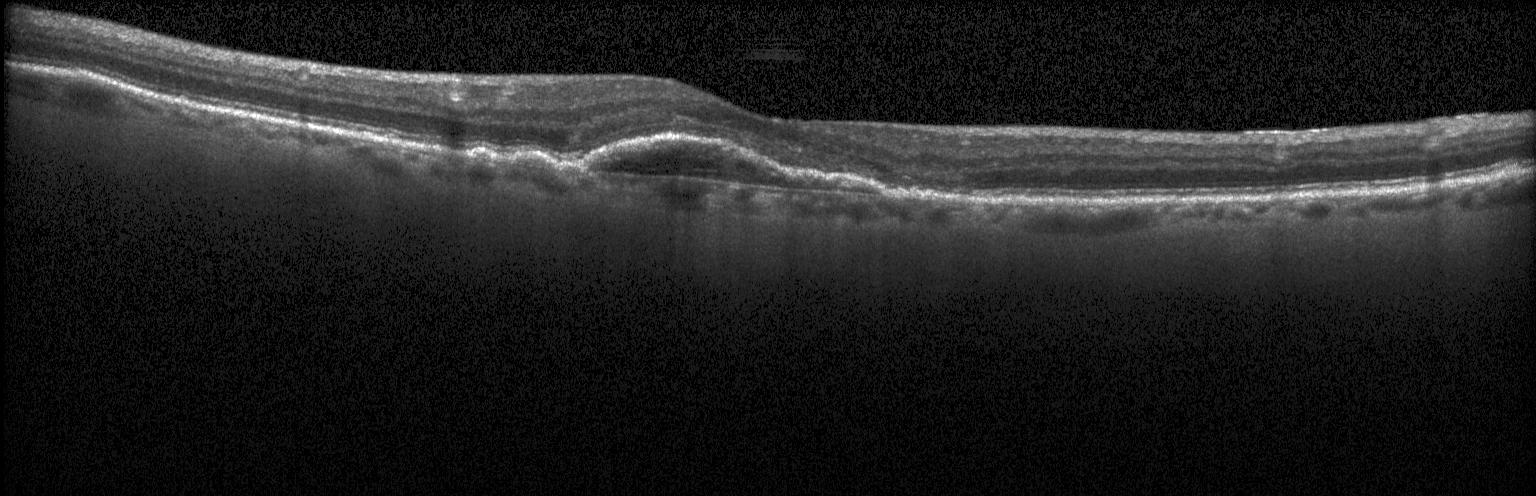
SD-OCT; optical coherence tomography B-scan; acquired on a Heidelberg Spectralis; centered on the fovea — Impression: a choroidal neovascular membrane.